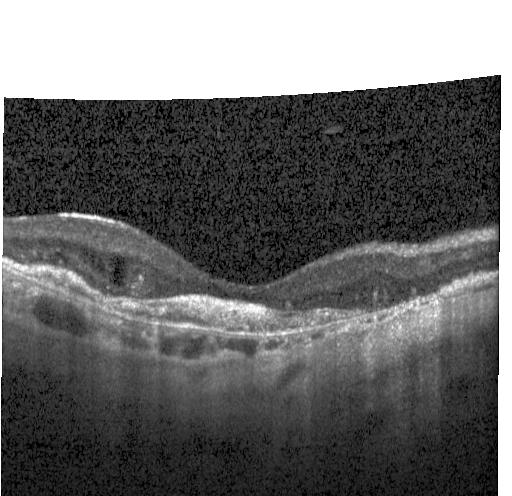

Finding: a choroidal neovascular membrane.